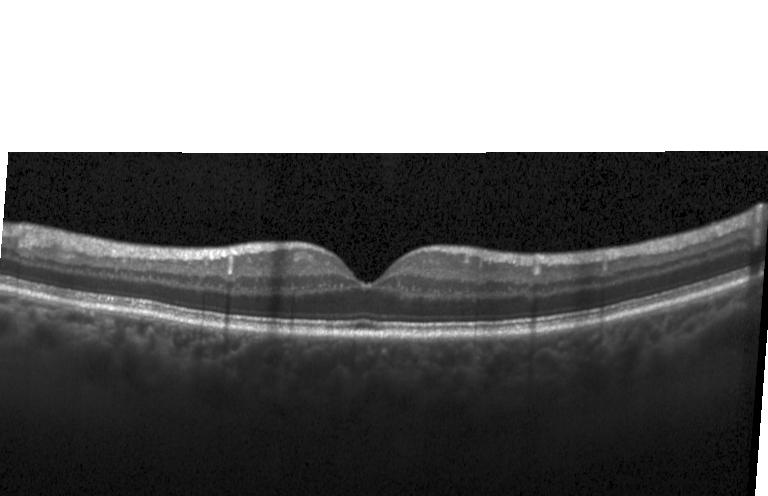

Retinal OCT cross-section showing neither choroidal neovascularization, diabetic macular edema, nor drusen.